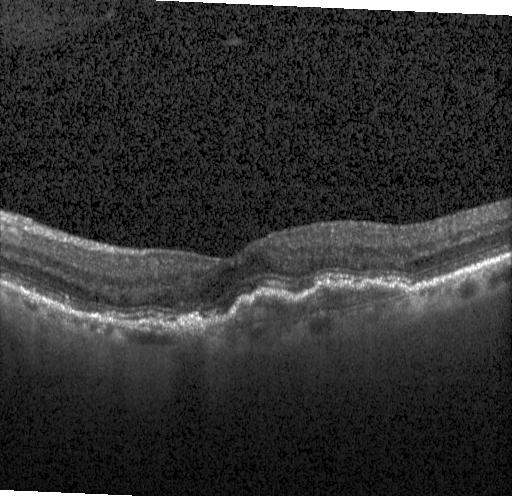
SD-OCT, optical coherence tomography B-scan, acquired on a Heidelberg Spectralis — Finding: choroidal neovascularization (CNV).